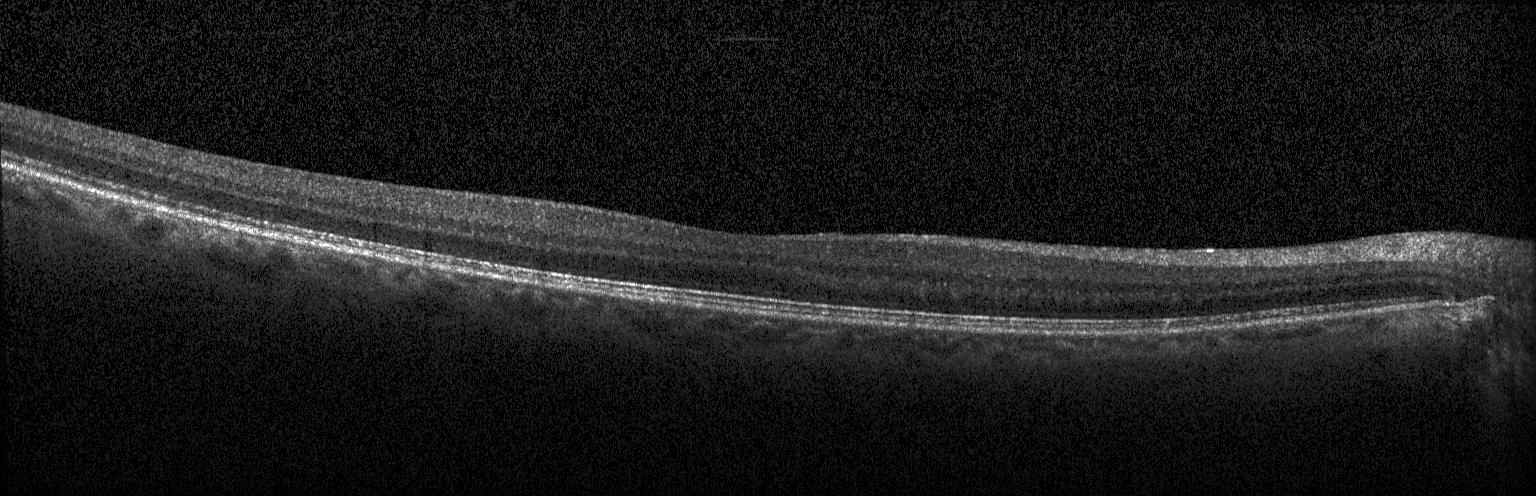
OCT B-scan showing no evidence of choroidal neovascularization, diabetic macular edema, or drusen.